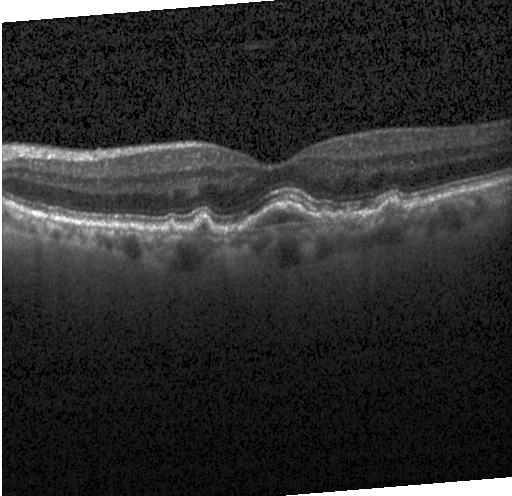
Assessment: choroidal neovascularization (CNV).